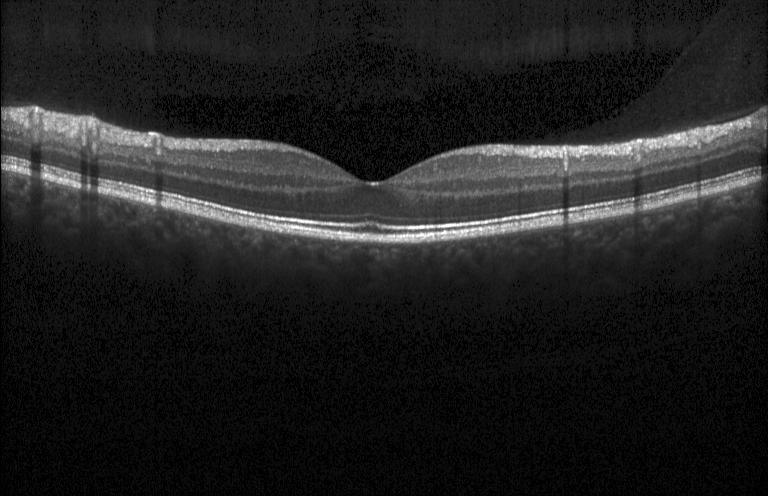 Retinal OCT cross-section, horizontal scan through the fovea. Finding: no choroidal neovascularization, diabetic macular edema, or drusen.